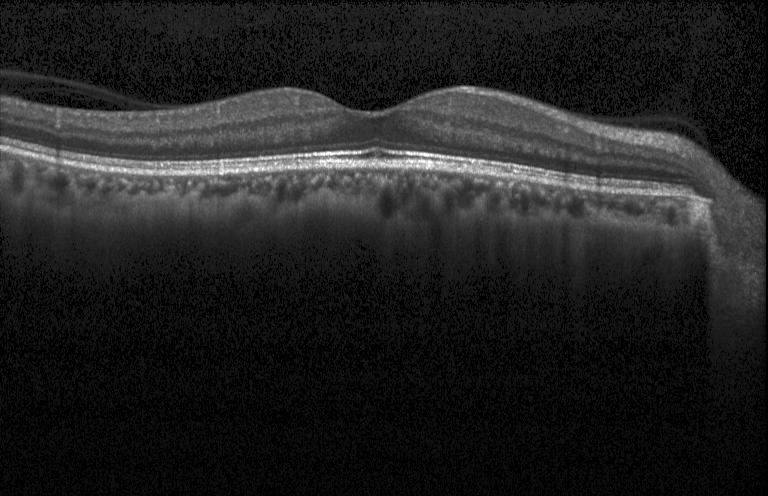

Dx: no choroidal neovascularization, diabetic macular edema, or drusen.